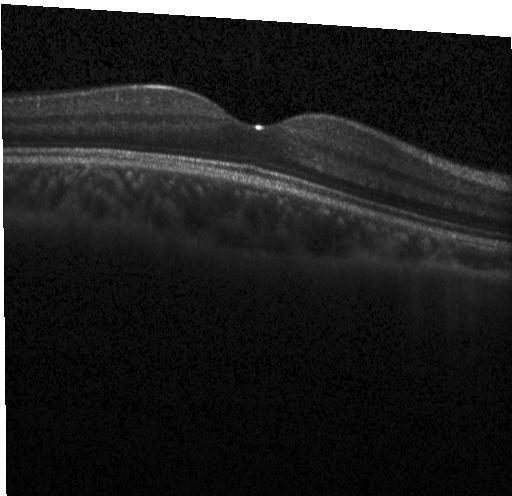
Spectral-domain optical coherence tomography. Through the macula. OCT B-scan
This B-scan demonstrates no choroidal neovascularization, no diabetic macular edema, and no drusen.